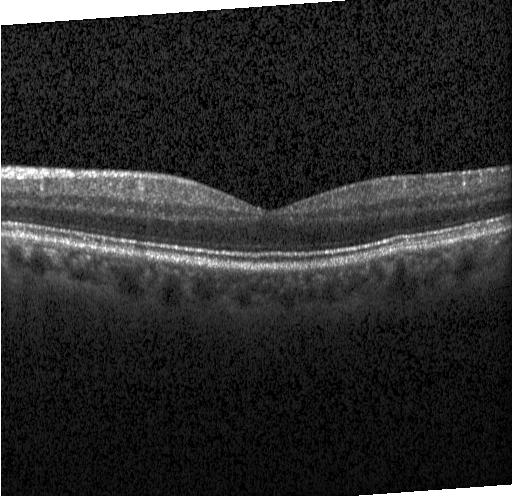
OCT B-scan · Heidelberg Spectralis · SD-OCT
Finding: no CNV, DME, or drusen.